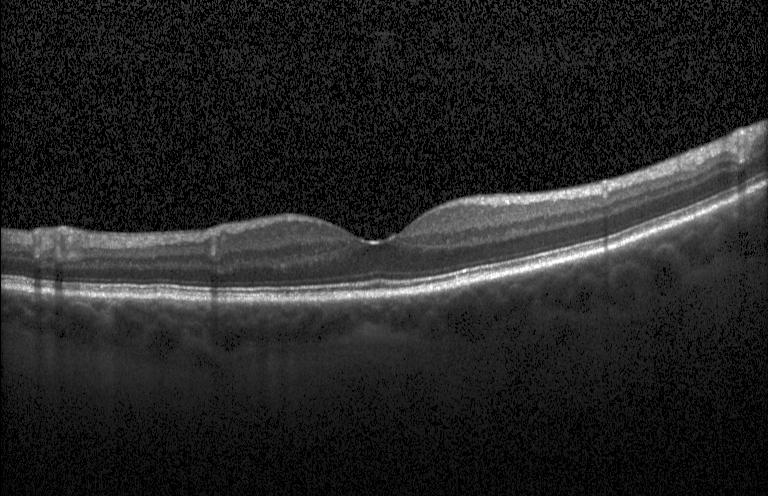 No choroidal neovascularization, no diabetic macular edema, and no drusen.